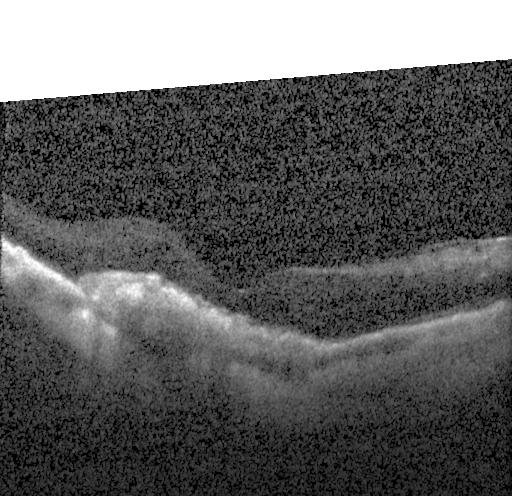

The scan shows choroidal neovascularization (CNV).